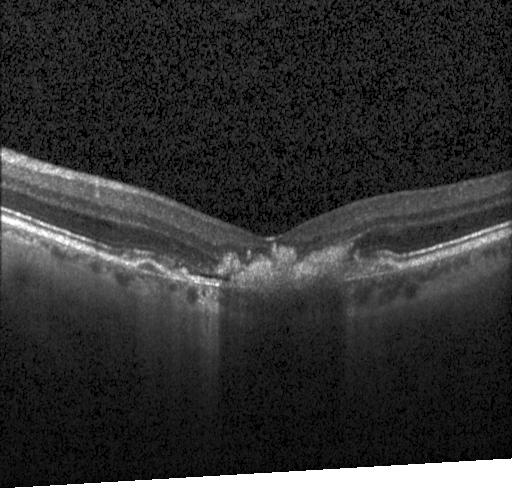

Retinal OCT cross-section.
Macular OCT: CNV.